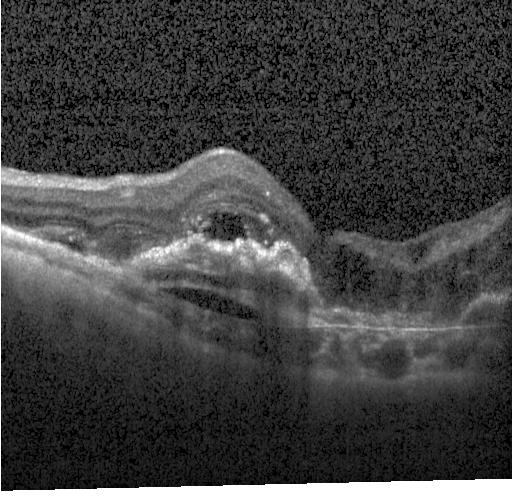

Assessment: choroidal neovascularization (CNV).